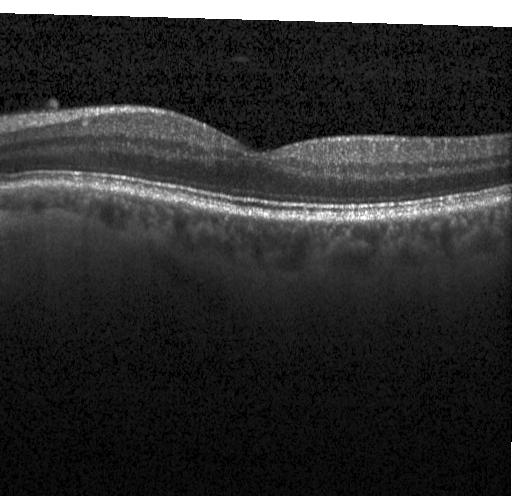 Instrument: Heidelberg Spectralis. OCT line scan. Macular OCT: no evidence of CNV, DME, or drusen.